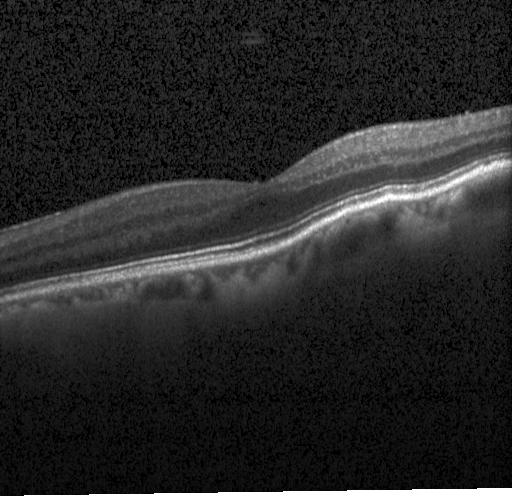
Horizontal scan through the fovea, acquired on a Heidelberg Spectralis, OCT line scan, SD-OCT. Impression: no choroidal neovascularization, diabetic macular edema, or drusen.